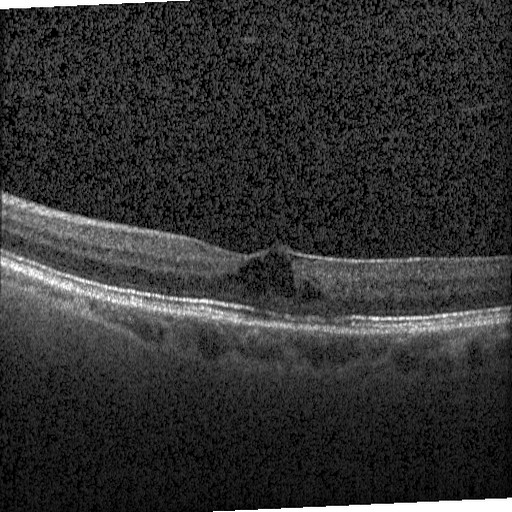 Optical coherence tomography scan.
OCT finding: diabetic macular edema.